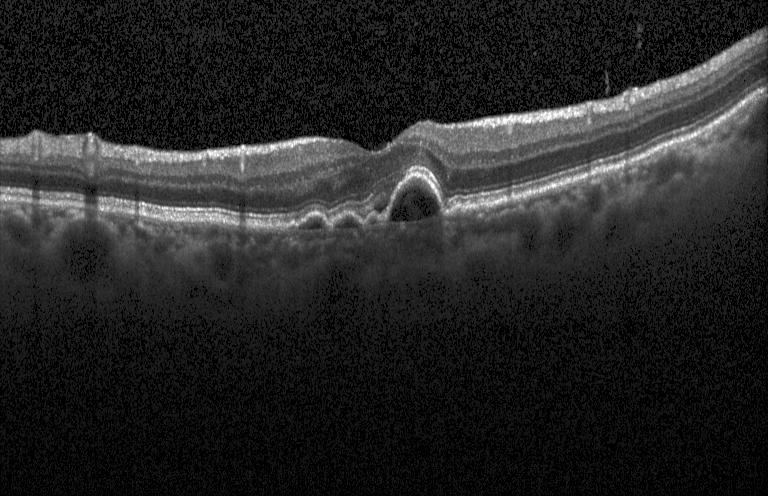

Choroidal neovascularization.